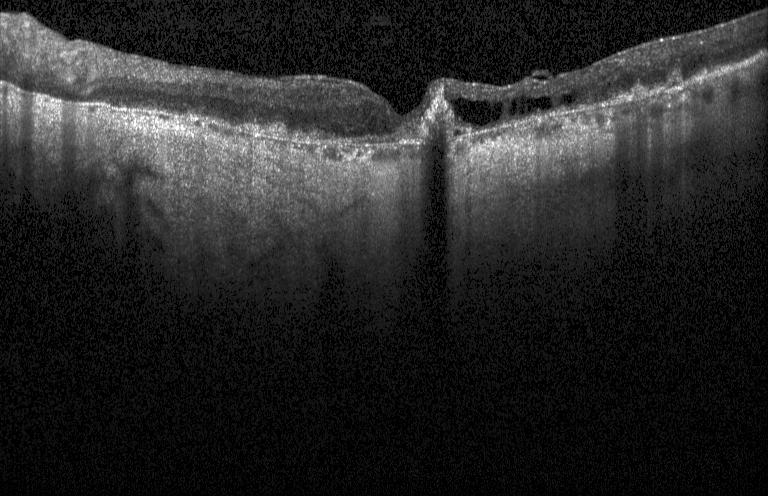 Fovea-centered; SD-OCT; retinal OCT cross-section; Heidelberg Spectralis. A choroidal neovascular membrane.